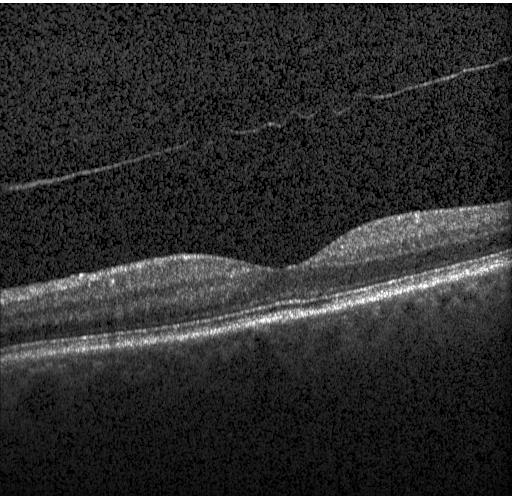

Heidelberg Spectralis OCT system · optical coherence tomography scan. Diagnosis: no evidence of CNV, DME, or drusen.